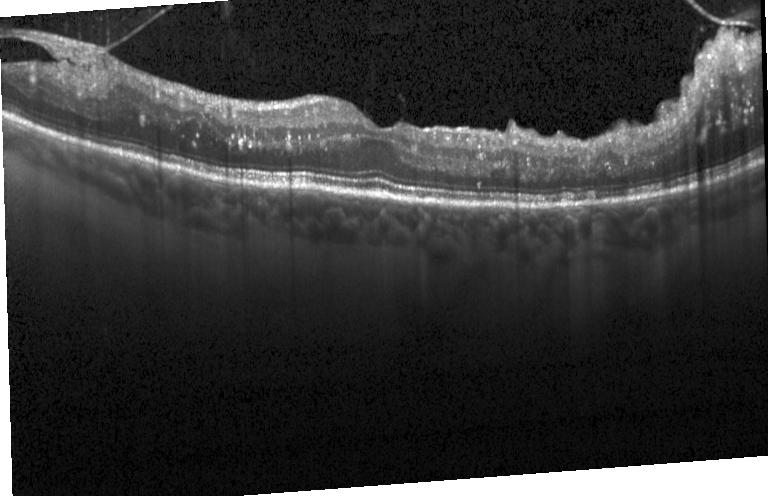
Macular scan. Acquired on a Heidelberg Spectralis. OCT B-scan. SD-OCT — Impression: diabetic macular edema (DME).